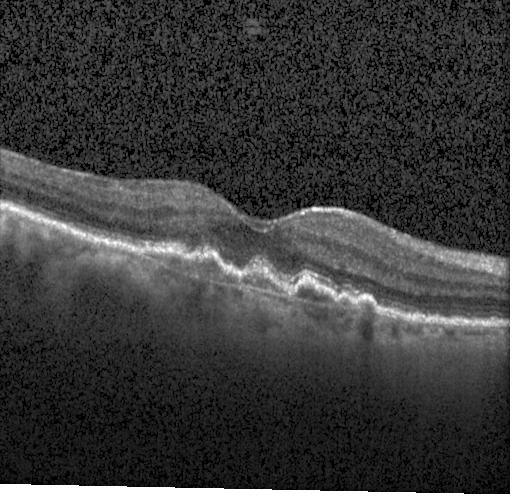

OCT line scan, spectral-domain OCT — Assessment: a choroidal neovascular membrane.